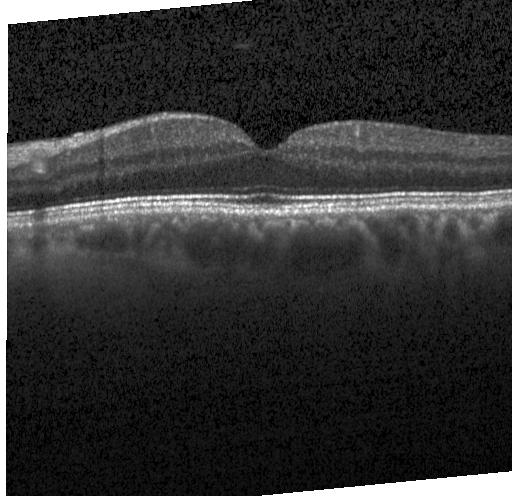
OCT line scan.
Macular OCT: no choroidal neovascularization, no diabetic macular edema, and no drusen.